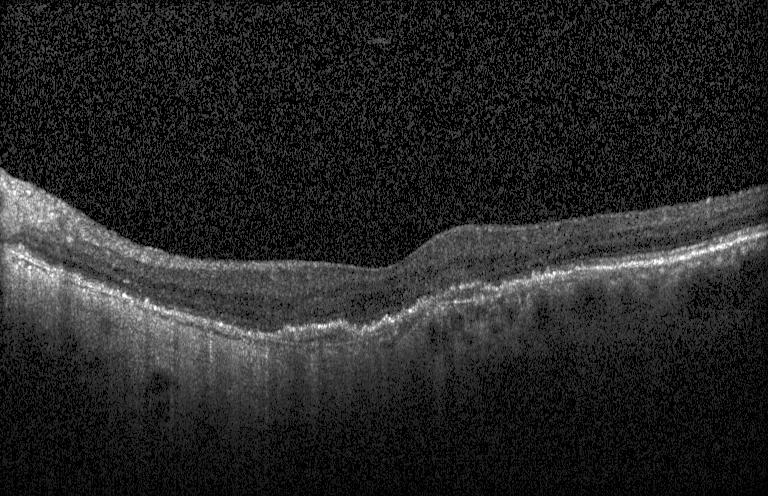

Retinal OCT cross-section.
Diagnosis: a choroidal neovascular membrane.